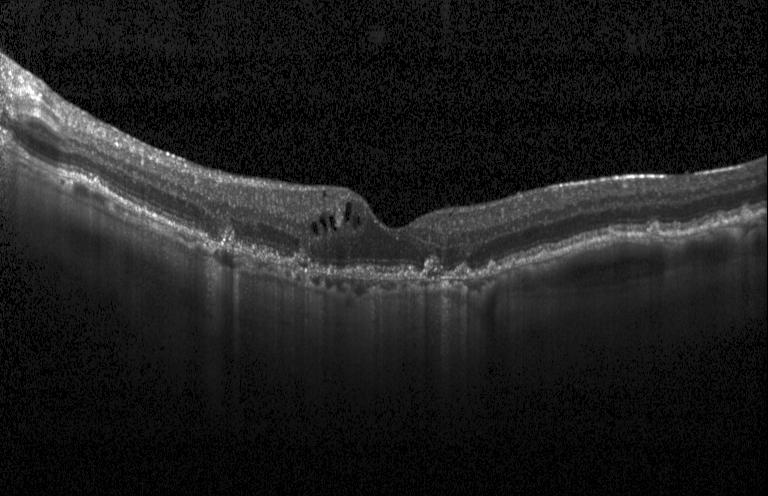
Macular OCT: a choroidal neovascular membrane.